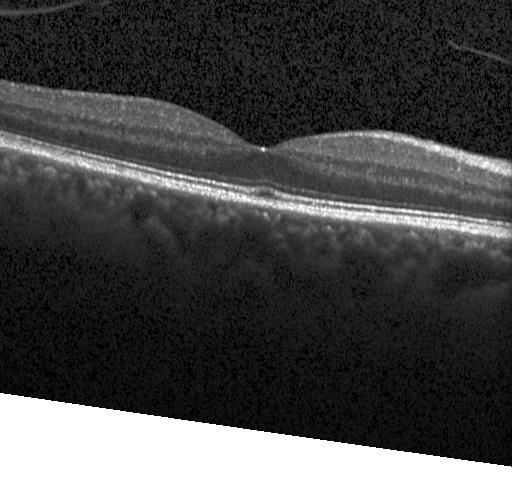

Impression: no choroidal neovascularization, diabetic macular edema, or drusen.